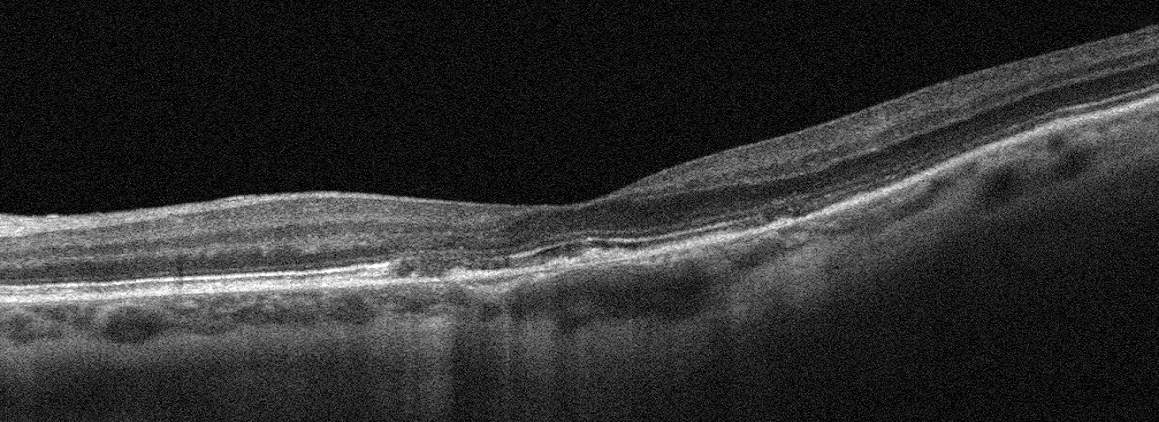
Oculus sinister. Optical coherence tomography scan. Diagnosis: age-related macular degeneration.